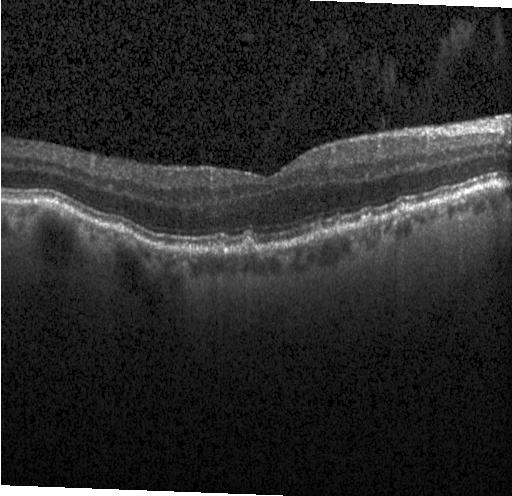

Spectral-domain OCT; optical coherence tomography B-scan; horizontal scan through the fovea; Heidelberg Spectralis — This B-scan demonstrates sub-RPE drusenoid deposits.